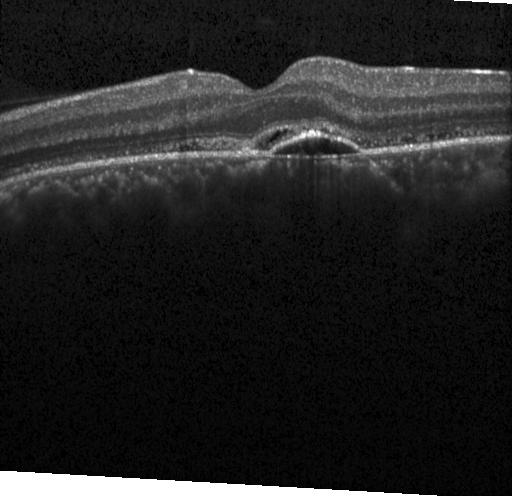
Retinal OCT cross-section
A choroidal neovascular membrane.